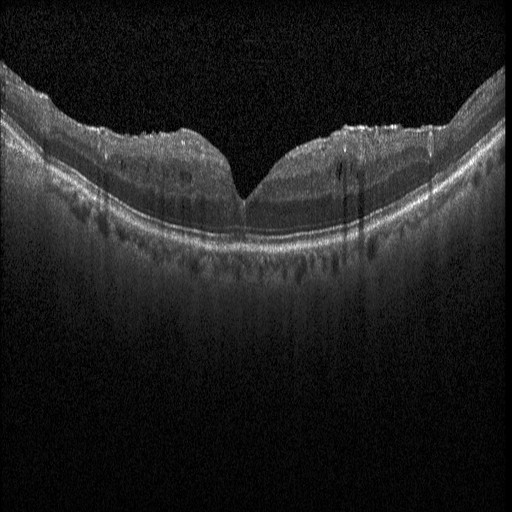

Macular OCT demonstrating DME.